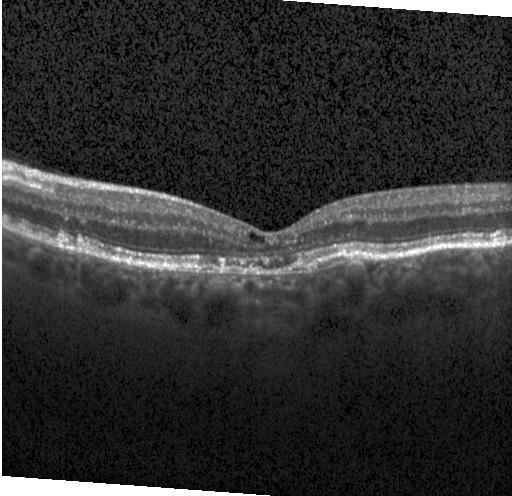
Impression: a choroidal neovascular membrane.